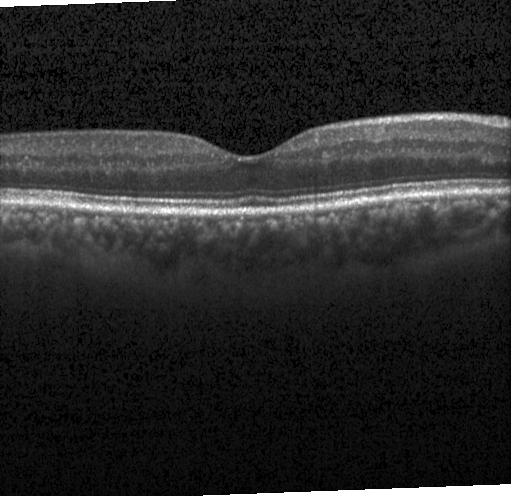
Optical coherence tomography B-scan — Assessment: no choroidal neovascularization, diabetic macular edema, or drusen.